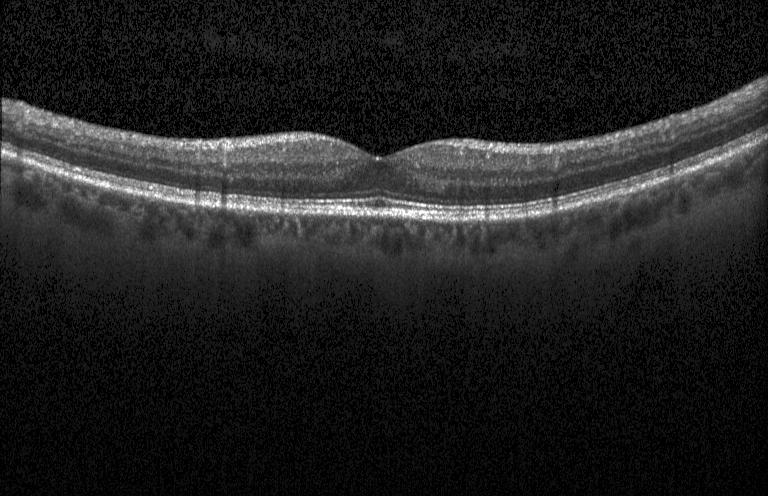

OCT B-scan showing no choroidal neovascularization, no diabetic macular edema, and no drusen.